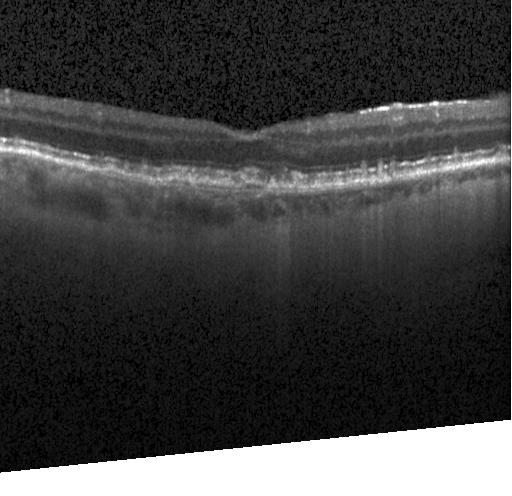

OCT finding: sub-RPE drusenoid deposits.